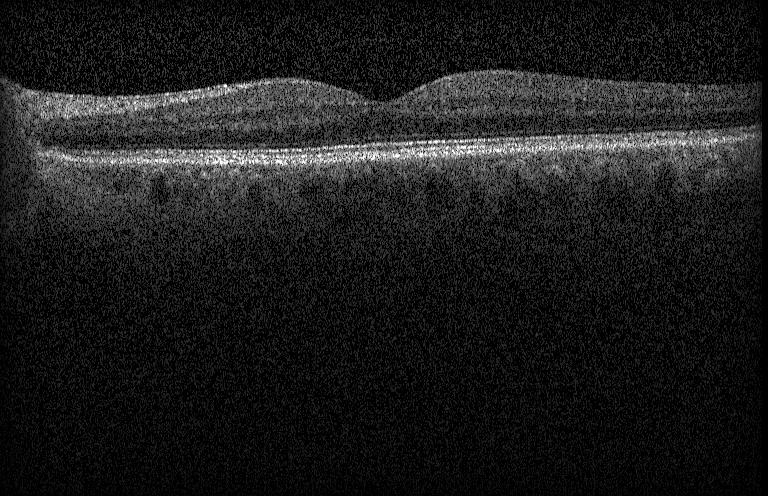
OCT B-scan. Through the macula. Acquired on a Heidelberg Spectralis. Spectral-domain optical coherence tomography — Dx: no choroidal neovascularization, diabetic macular edema, or drusen.